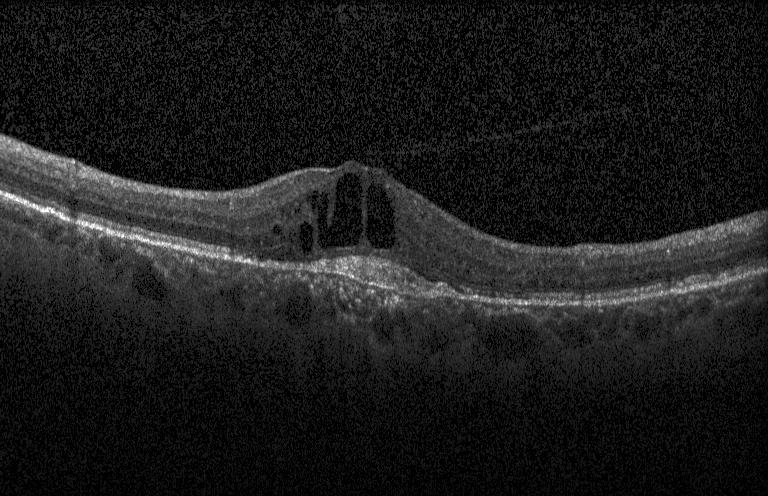

Instrument: Heidelberg Spectralis. Retinal OCT B-scan. Spectral-domain OCT
This B-scan demonstrates choroidal neovascularization.